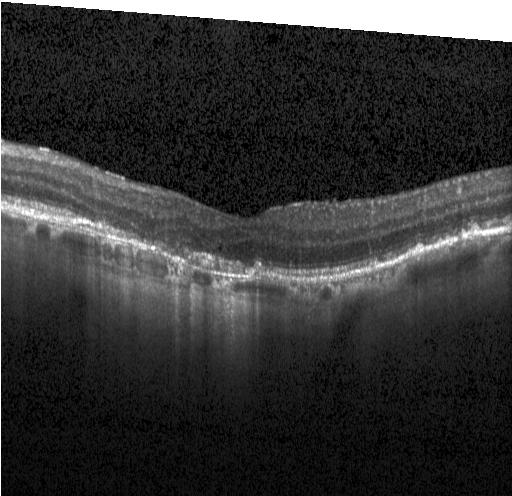
OCT B-scan · horizontal scan through the fovea · Heidelberg Spectralis OCT system. This B-scan demonstrates no choroidal neovascularization, no diabetic macular edema, and no drusen.